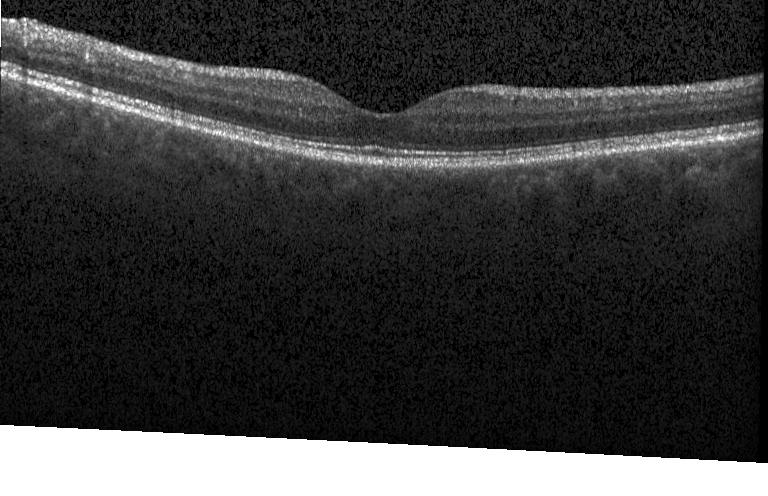

Assessment: neither CNV, DME, nor drusen.